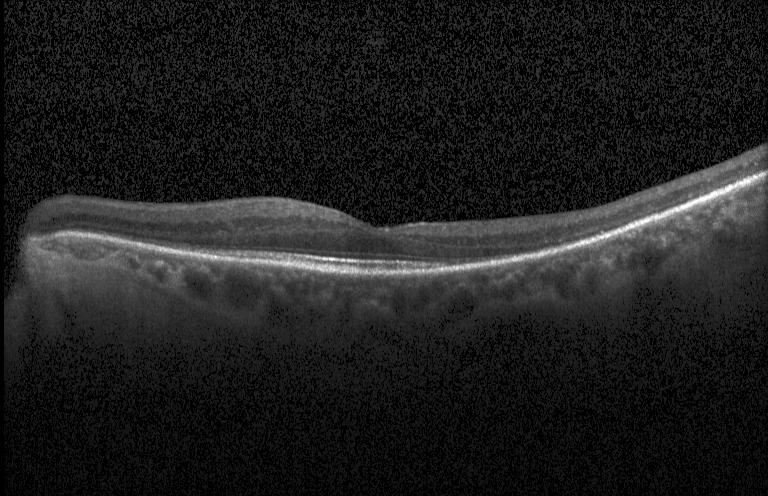
Optical coherence tomography scan, centered on the fovea.
Assessment: no choroidal neovascularization, no diabetic macular edema, and no drusen.